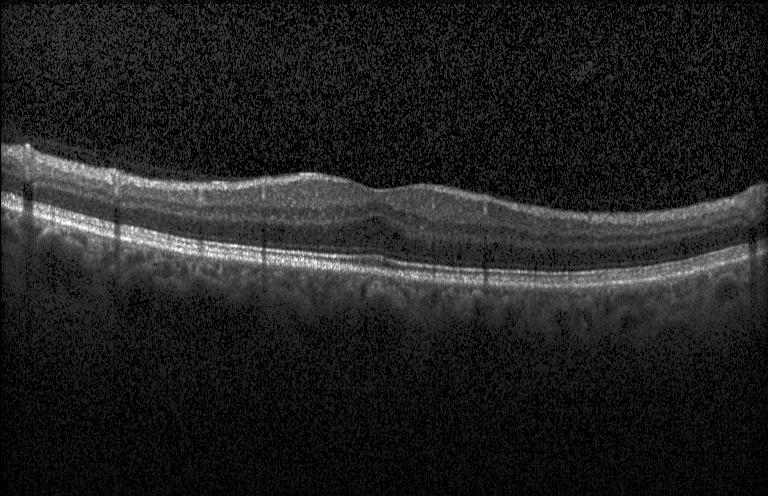

Retinal OCT cross-section, fovea-centered, instrument: Heidelberg Spectralis. No evidence of CNV, DME, or drusen.